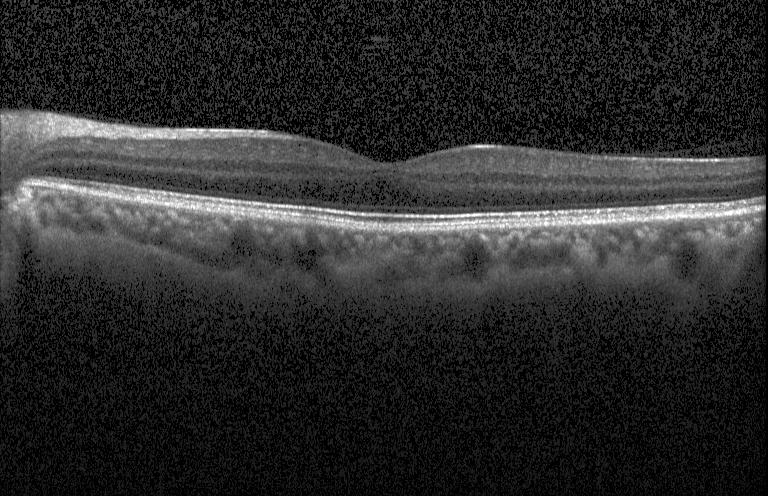 SD-OCT. Heidelberg Spectralis. Optical coherence tomography B-scan — Diagnosis: no evidence of choroidal neovascularization, diabetic macular edema, or drusen.